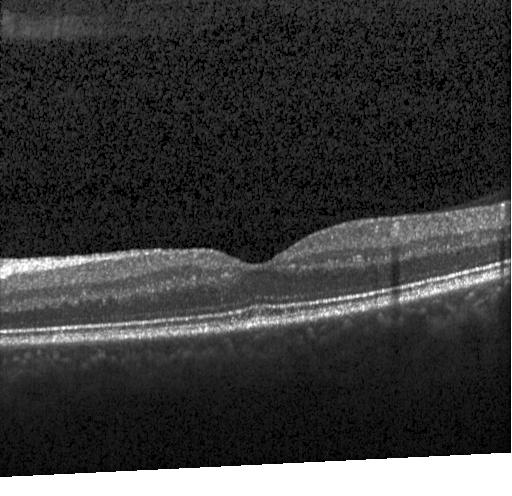

Spectral-domain optical coherence tomography. Heidelberg Spectralis. OCT B-scan.
This B-scan demonstrates no evidence of choroidal neovascularization, diabetic macular edema, or drusen.